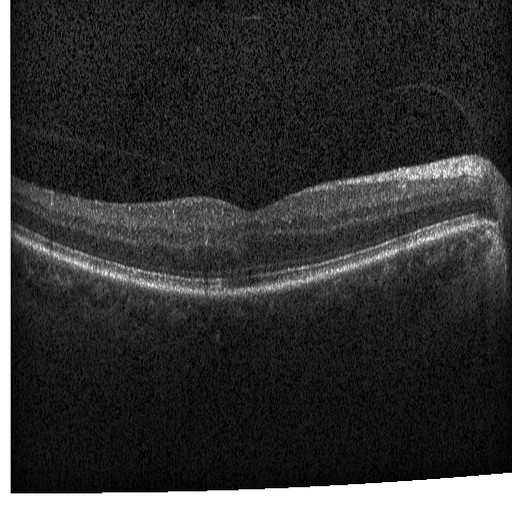
Retinal OCT cross-section.
Macular OCT: DME.